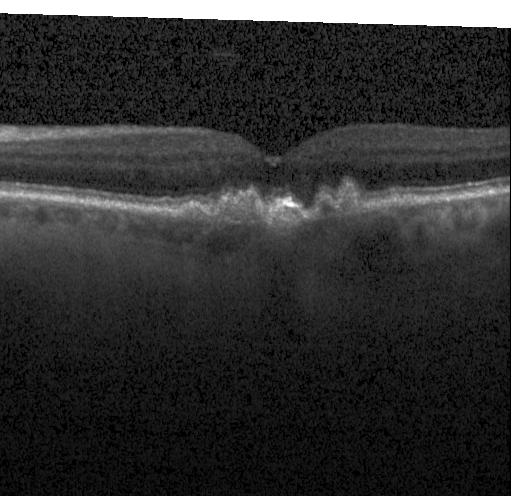
CNV.